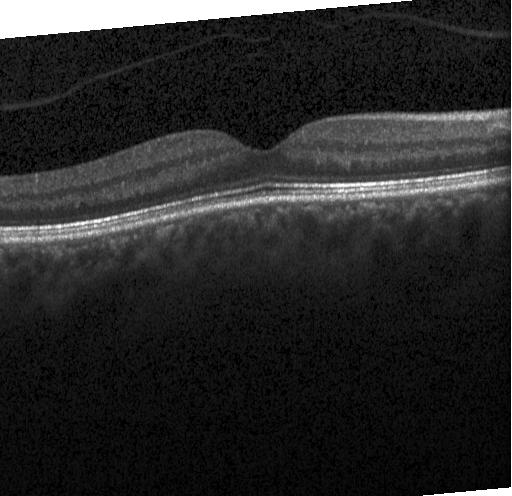
OCT B-scan.
Finding: no CNV, DME, or drusen.